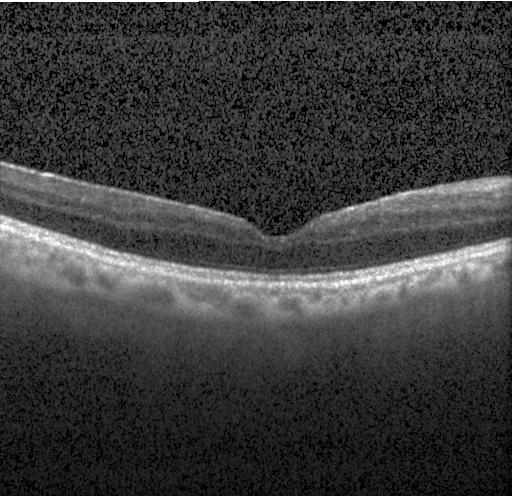 OCT B-scan.
Macular OCT: no choroidal neovascularization, no diabetic macular edema, and no drusen.